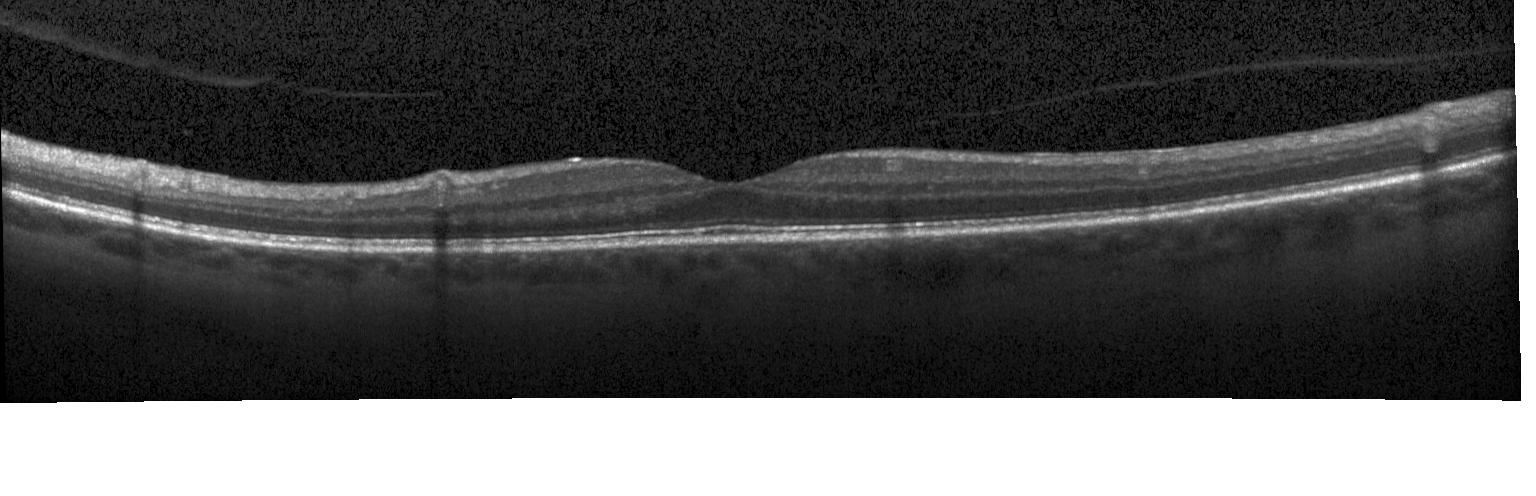

Optical coherence tomography B-scan. The scan shows no CNV, DME, or drusen.